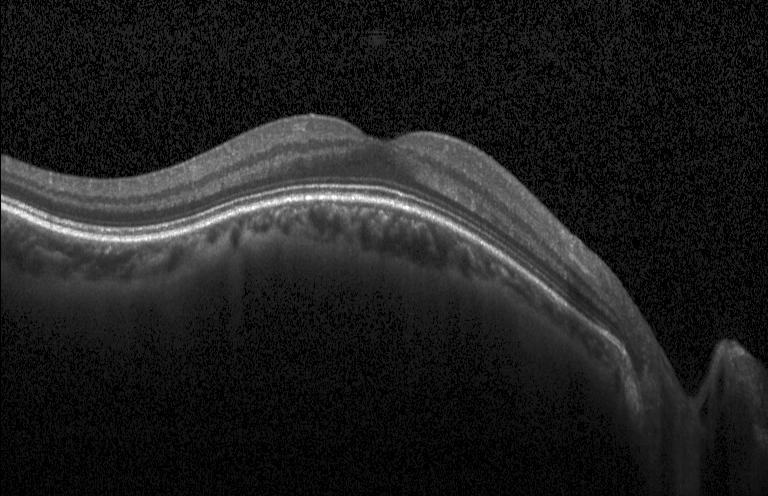

Macular OCT demonstrating no choroidal neovascularization, diabetic macular edema, or drusen.